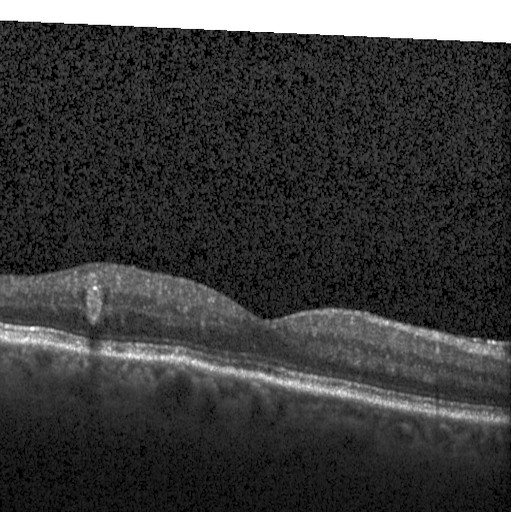 OCT B-scan · fovea-centered. Impression: diabetic macular edema (DME).